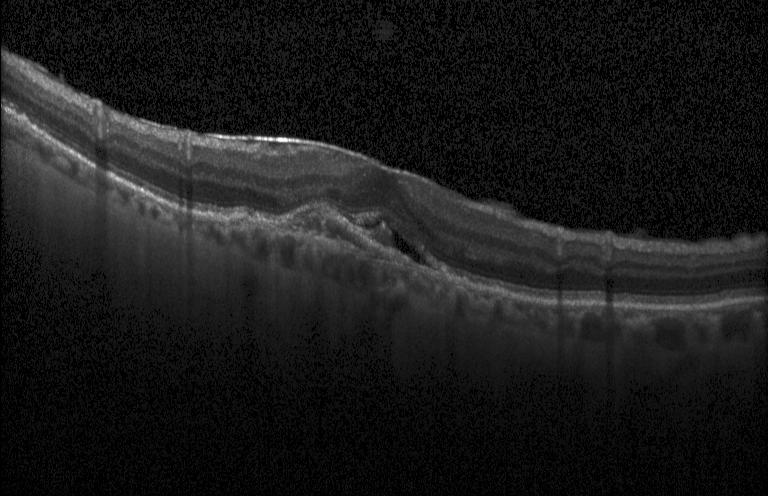

Macular OCT: CNV.